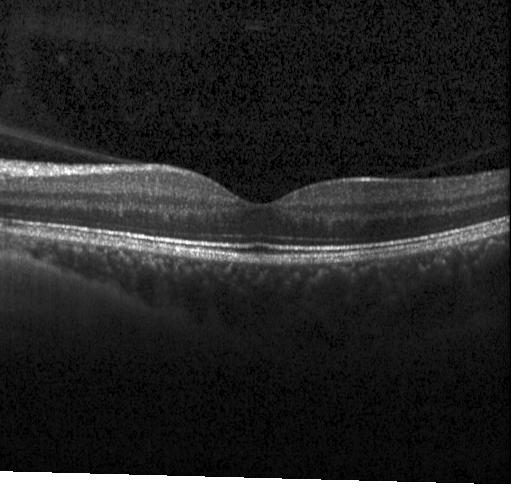

Spectral-domain OCT B-scan: neither choroidal neovascularization, diabetic macular edema, nor drusen.